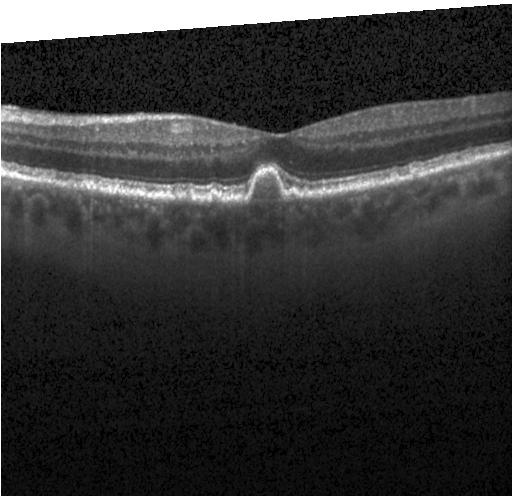 Optical coherence tomography scan; through the macula
Finding: sub-RPE drusenoid deposits.